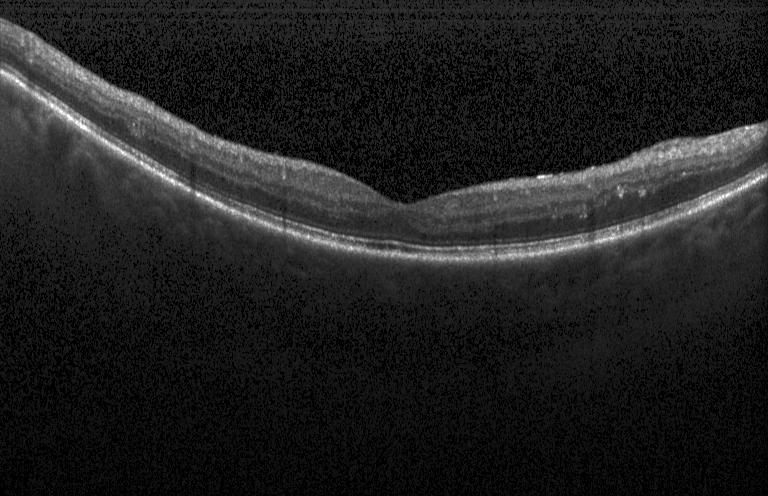 Acquired on a Heidelberg Spectralis, through the macula, spectral-domain OCT, optical coherence tomography scan — Assessment: no choroidal neovascularization, diabetic macular edema, or drusen.